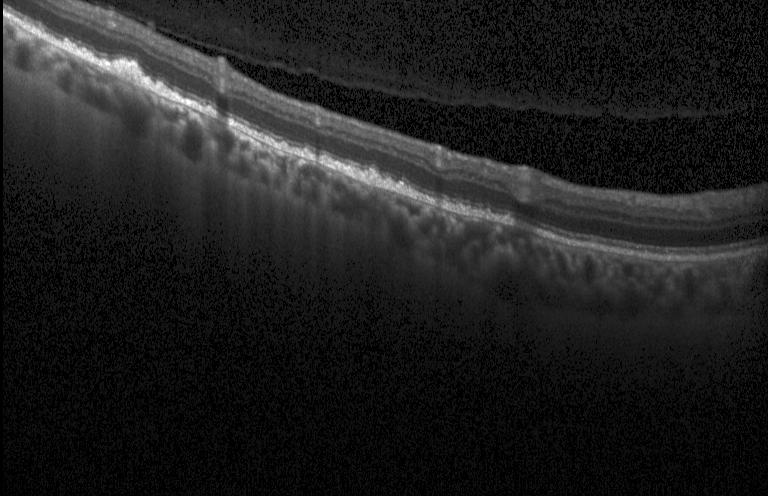

OCT scan showing sub-RPE drusenoid deposits.